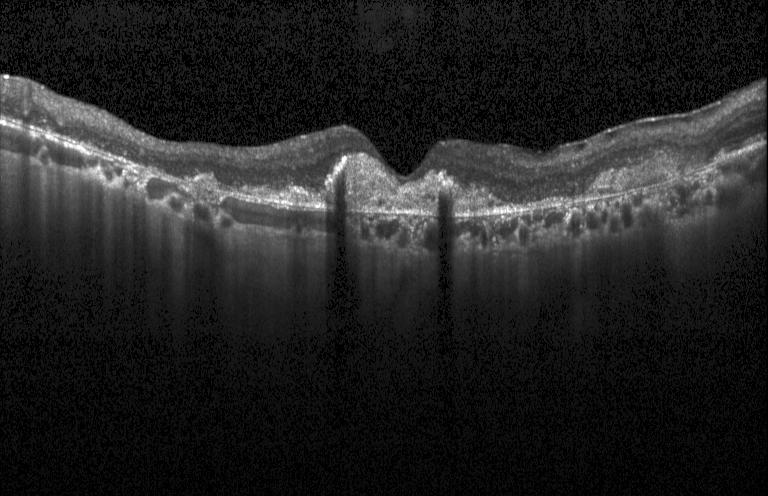

Heidelberg Spectralis OCT system · spectral-domain optical coherence tomography · retinal OCT B-scan — This B-scan demonstrates a choroidal neovascular membrane.